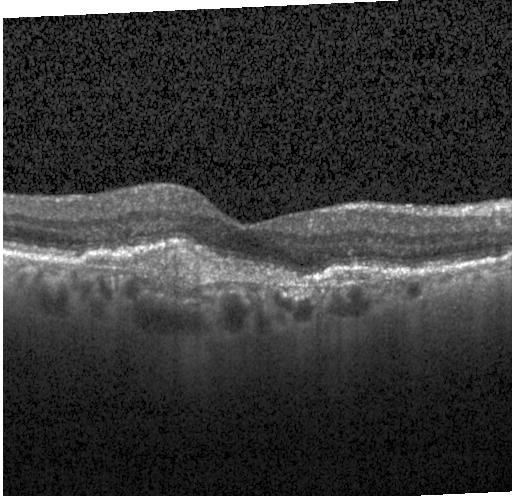

Retinal OCT cross-section; horizontal scan through the fovea; Heidelberg Spectralis; spectral-domain OCT
Impression: CNV.